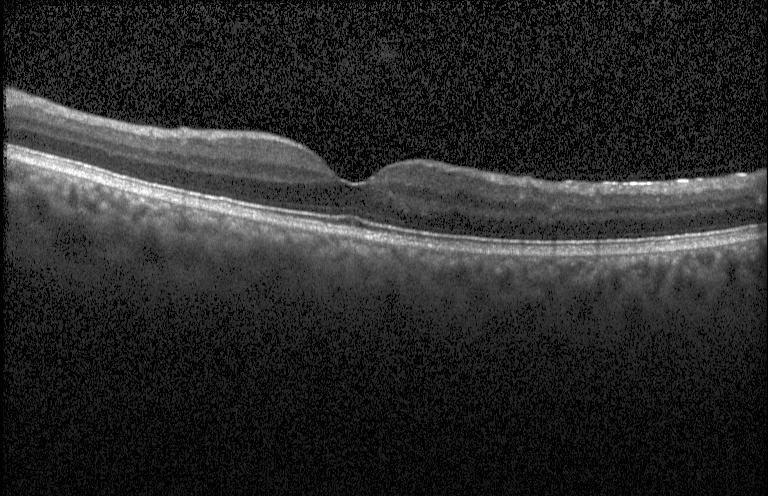

Acquired on a Heidelberg Spectralis, spectral-domain optical coherence tomography, through the macula, OCT B-scan
No evidence of CNV, DME, or drusen.